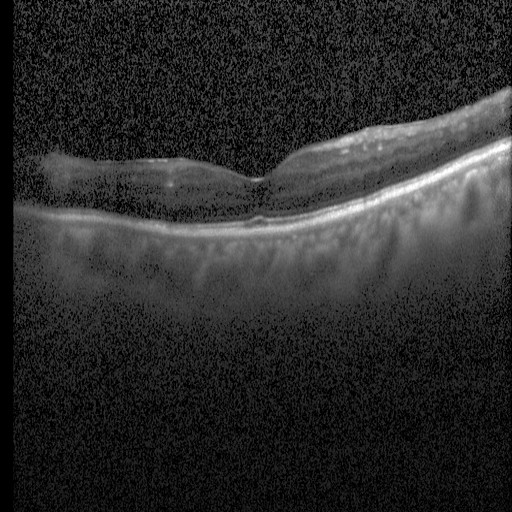
This B-scan demonstrates DME.